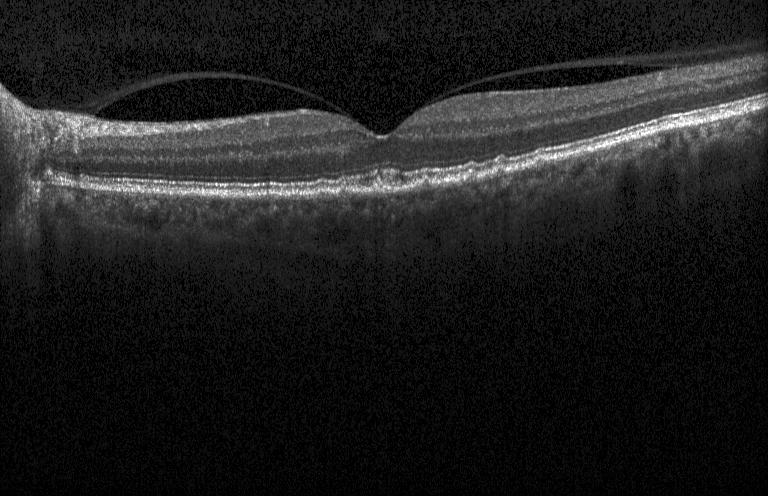

Diagnosis: drusen.